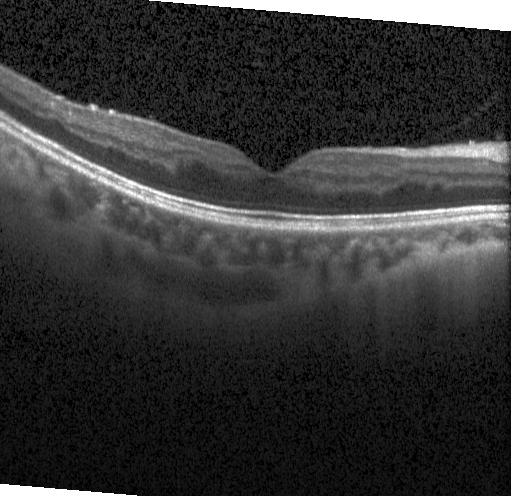

This B-scan demonstrates no choroidal neovascularization, no diabetic macular edema, and no drusen.